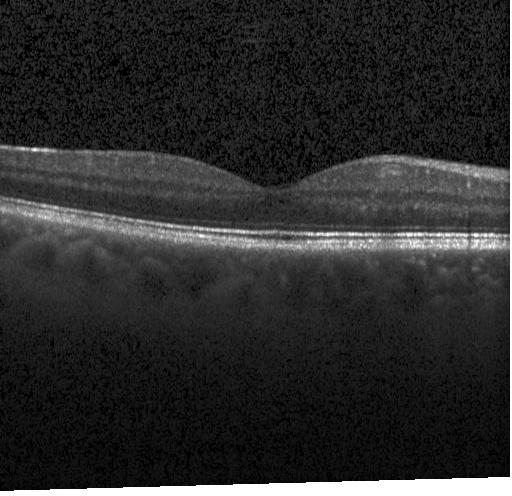

Impression: neither CNV, DME, nor drusen.